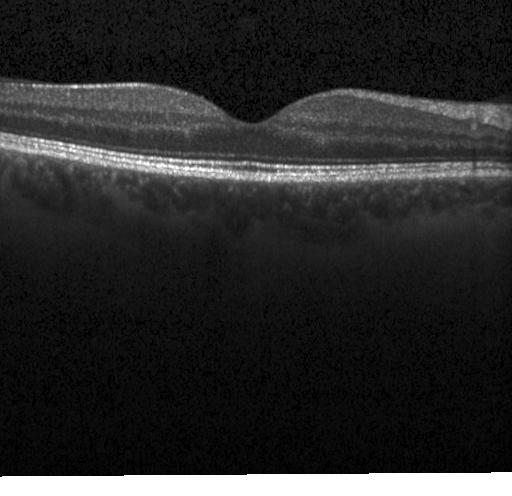
OCT finding: no evidence of choroidal neovascularization, diabetic macular edema, or drusen.